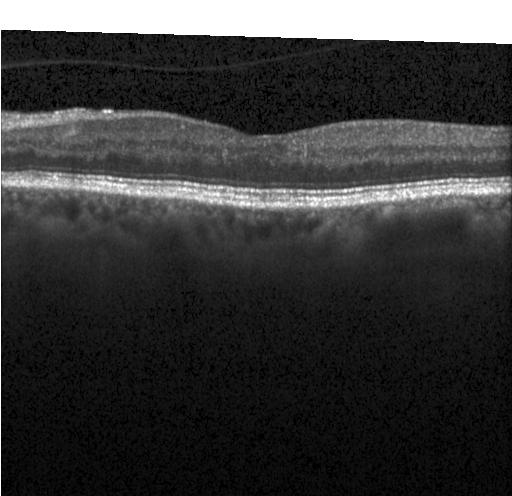
Optical coherence tomography B-scan
Finding: neither CNV, DME, nor drusen.